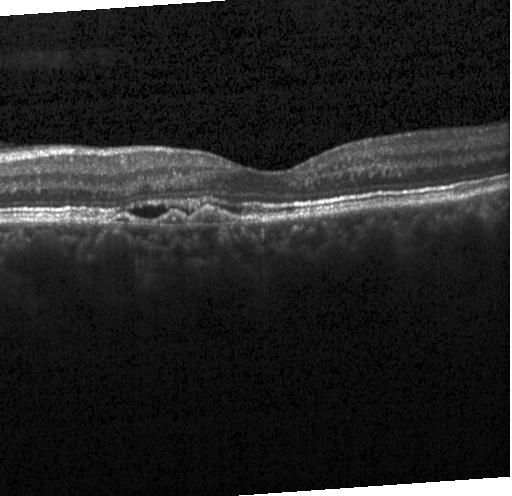

Fovea-centered; retinal OCT cross-section; Heidelberg Spectralis
Assessment: a choroidal neovascular membrane.